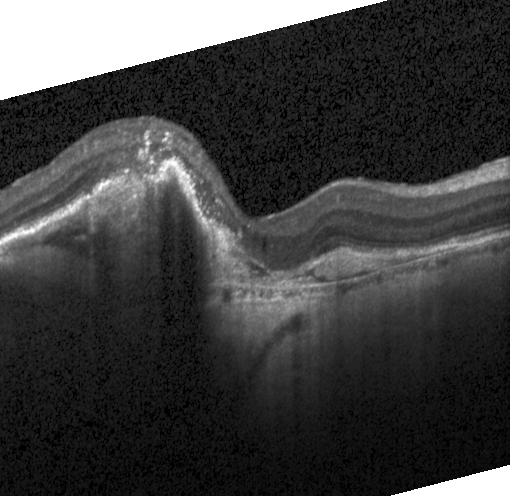
OCT line scan; Heidelberg Spectralis — A choroidal neovascular membrane.